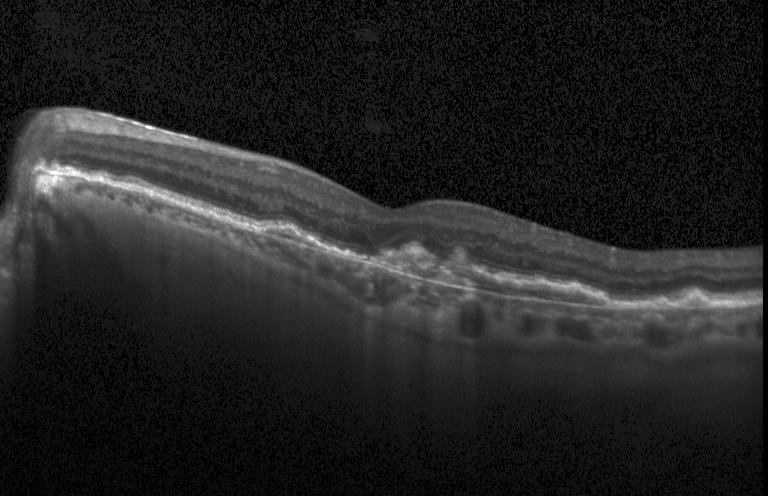
Heidelberg Spectralis OCT system; spectral-domain OCT; OCT line scan. This B-scan demonstrates a choroidal neovascular membrane.